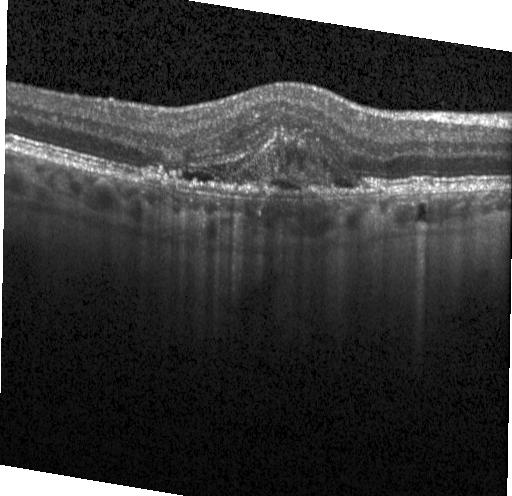 Horizontal scan through the fovea, acquired on a Heidelberg Spectralis, retinal OCT B-scan — A choroidal neovascular membrane.